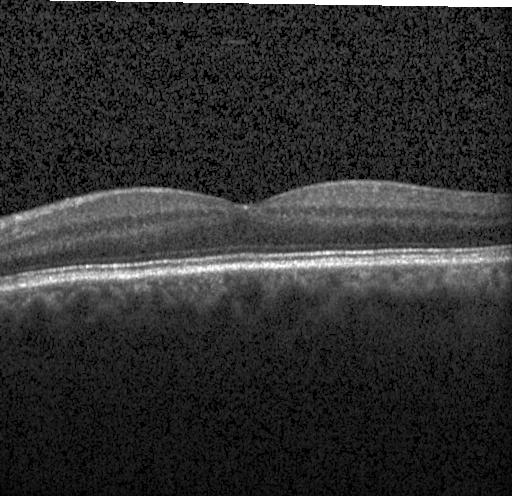

SD-OCT · centered on the fovea · retinal OCT cross-section · Heidelberg Spectralis
No choroidal neovascularization, diabetic macular edema, or drusen.